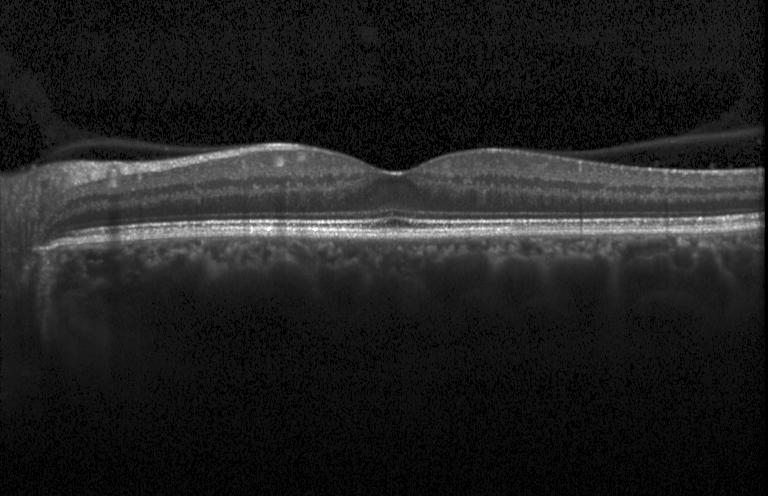 Centered on the fovea, spectral-domain OCT, optical coherence tomography scan.
Finding: no choroidal neovascularization, no diabetic macular edema, and no drusen.